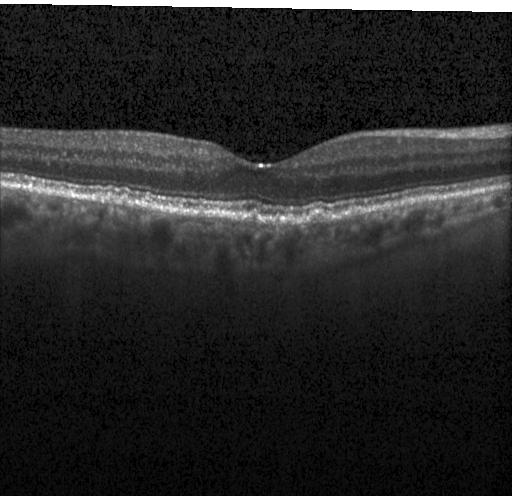 OCT B-scan · macular scan — Multiple drusen.